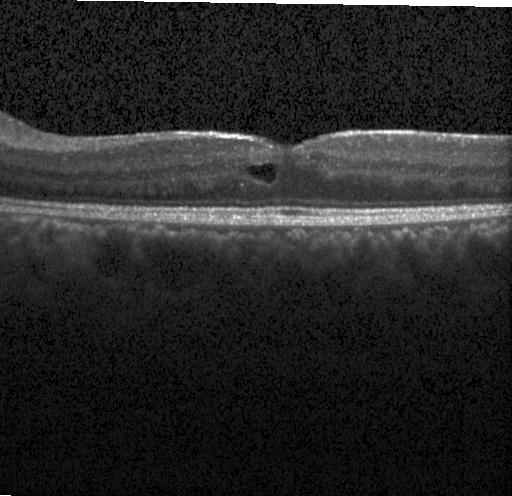
This B-scan demonstrates diabetic macular edema (DME).